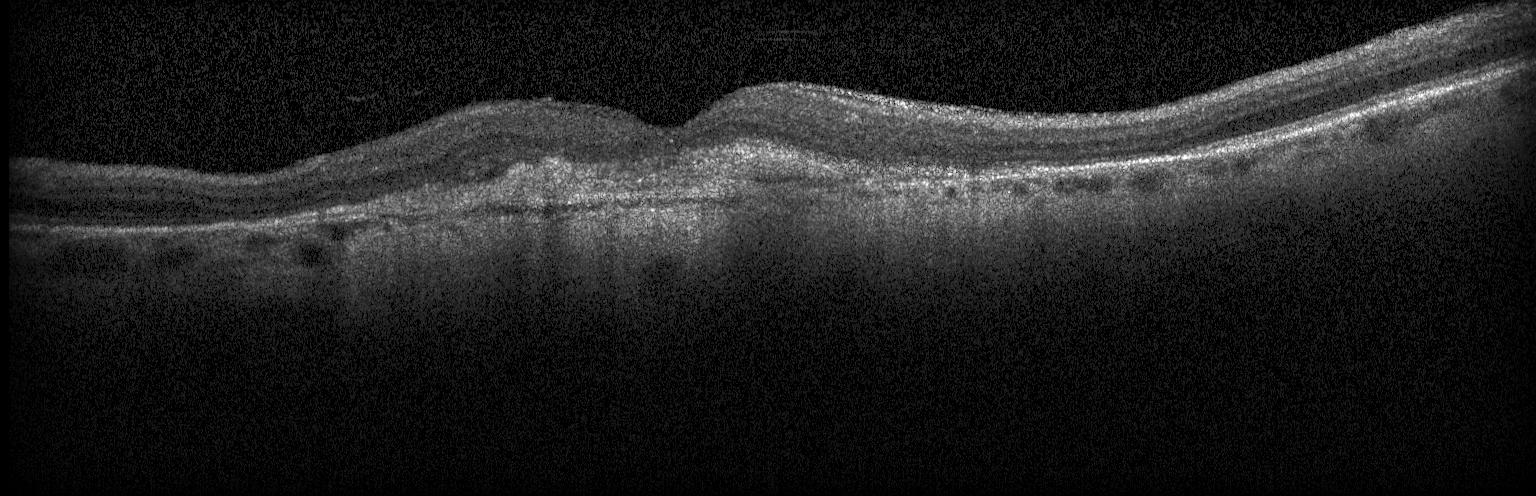

Macular scan; retinal OCT B-scan — Diagnosis: CNV.